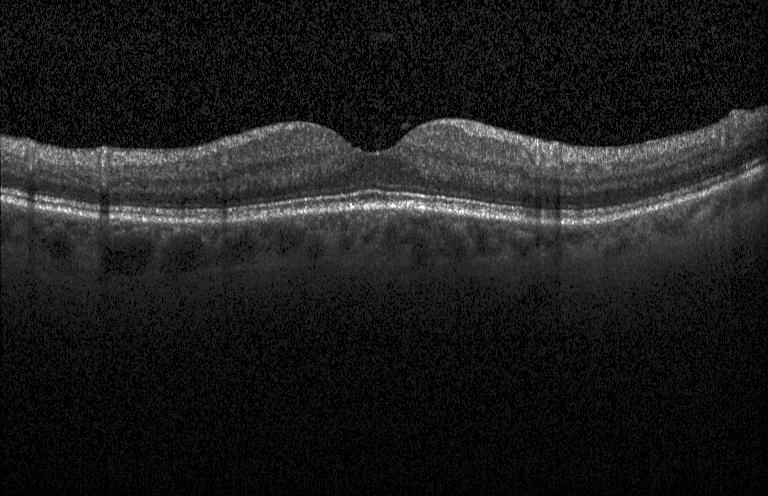 Macular scan. Heidelberg Spectralis OCT system. Spectral-domain optical coherence tomography. Retinal OCT cross-section.
Diagnosis: no choroidal neovascularization, diabetic macular edema, or drusen.